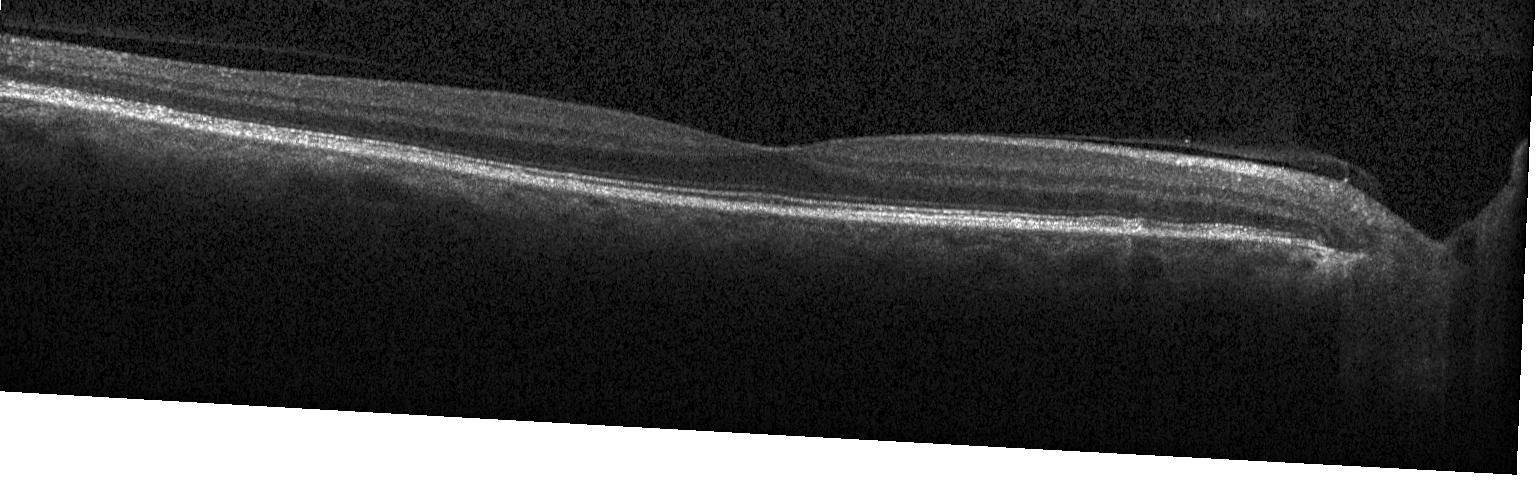 Optical coherence tomography B-scan. Fovea-centered.
Finding: no CNV, no DME, and no drusen.